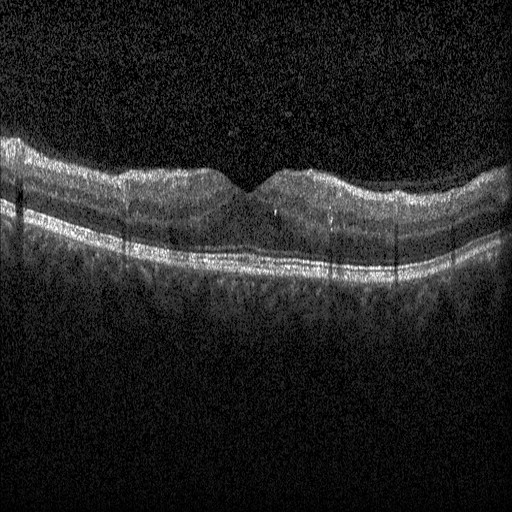 Centered on the fovea; optical coherence tomography B-scan. OCT finding: diabetic macular edema (DME).